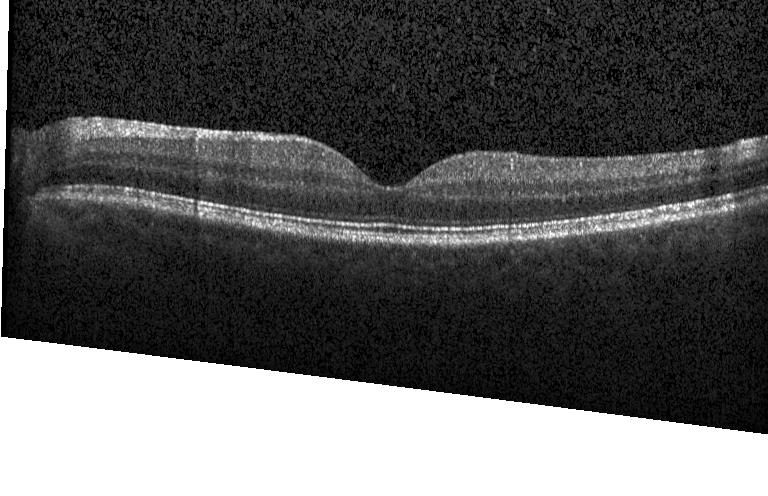 Retinal OCT cross-section, macular scan.
OCT finding: no evidence of CNV, DME, or drusen.